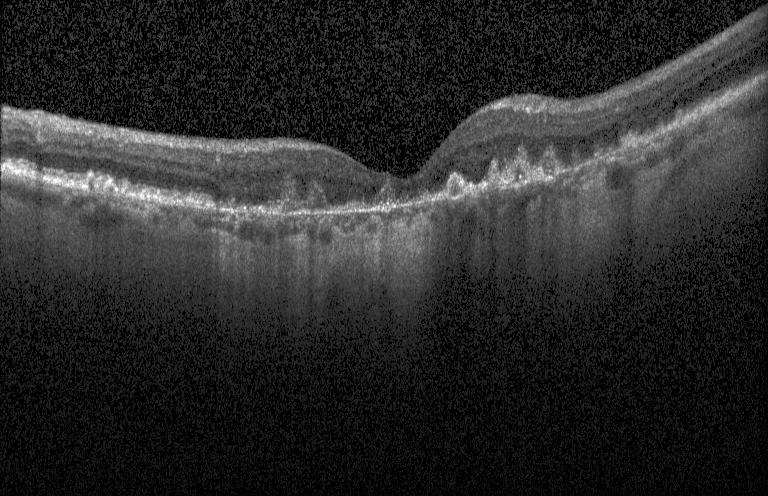
Heidelberg Spectralis. Retinal OCT B-scan. Diagnosis: CNV.